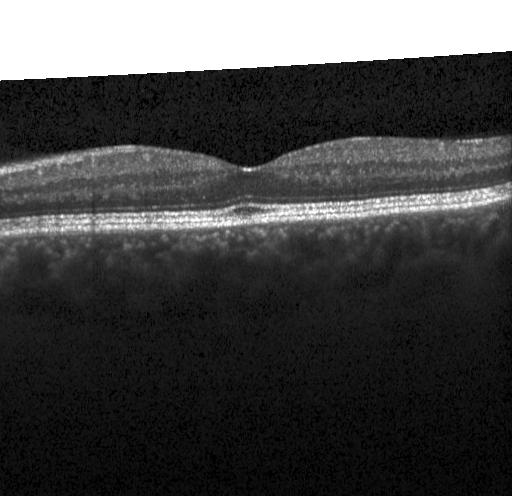
Macular OCT demonstrating neither CNV, DME, nor drusen.